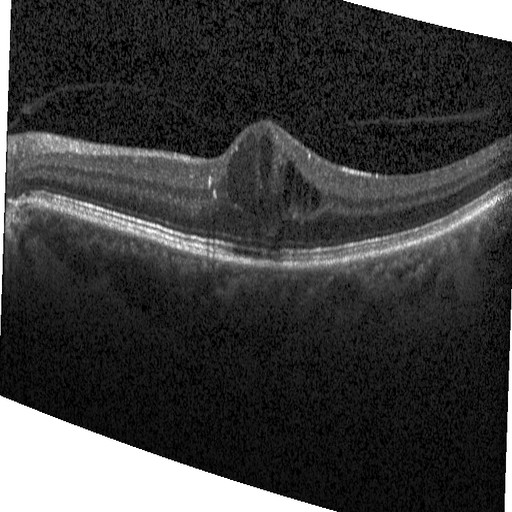 Dx: DME.